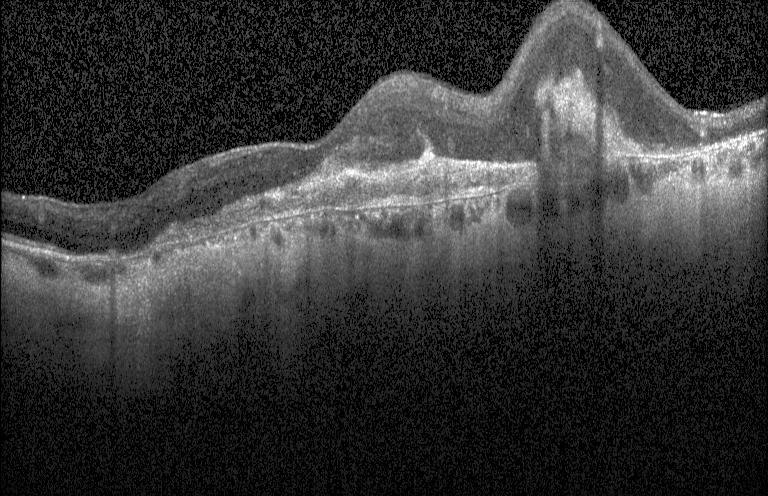

Retinal OCT B-scan. Diagnosis: choroidal neovascularization.